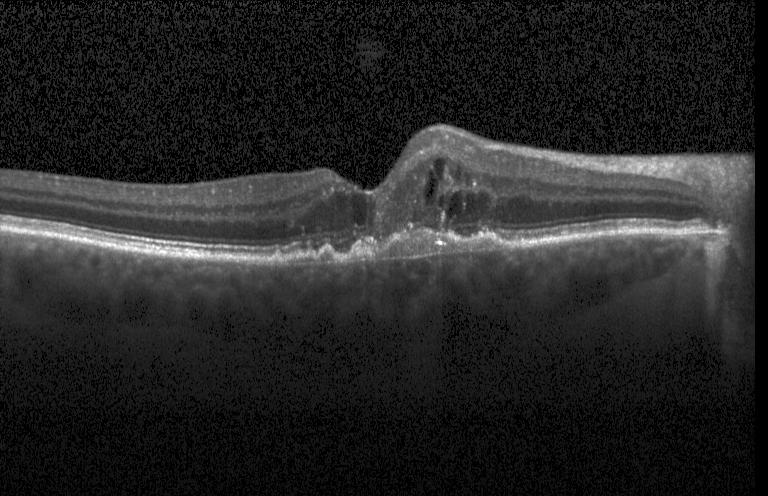
Optical coherence tomography scan, fovea-centered. Impression: a choroidal neovascular membrane.